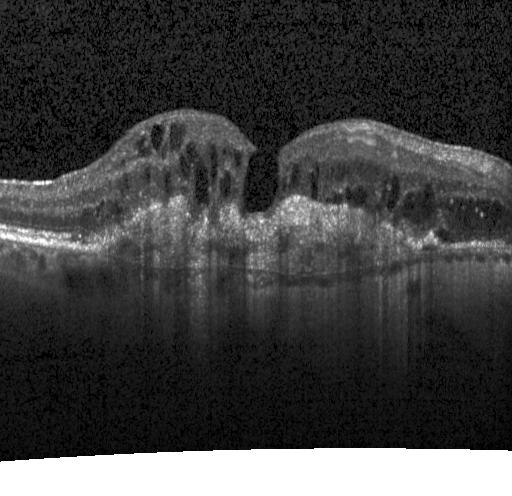

SD-OCT · Heidelberg Spectralis OCT system · optical coherence tomography B-scan · through the macula. Assessment: a choroidal neovascular membrane.